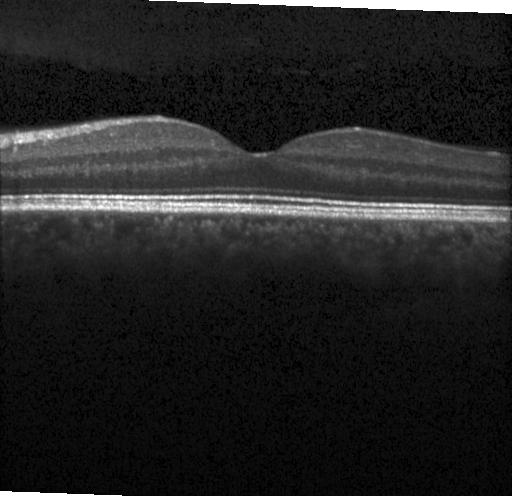 Optical coherence tomography scan · spectral-domain OCT.
No CNV, no DME, and no drusen.